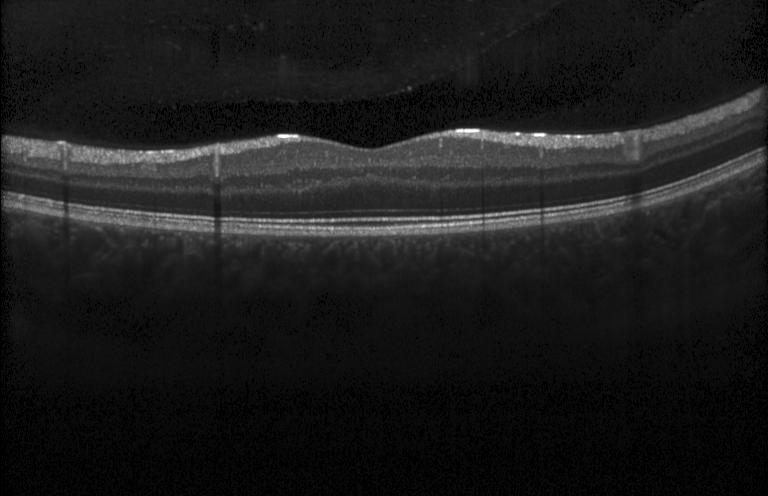
Fovea-centered · optical coherence tomography B-scan
OCT finding: no choroidal neovascularization, diabetic macular edema, or drusen.